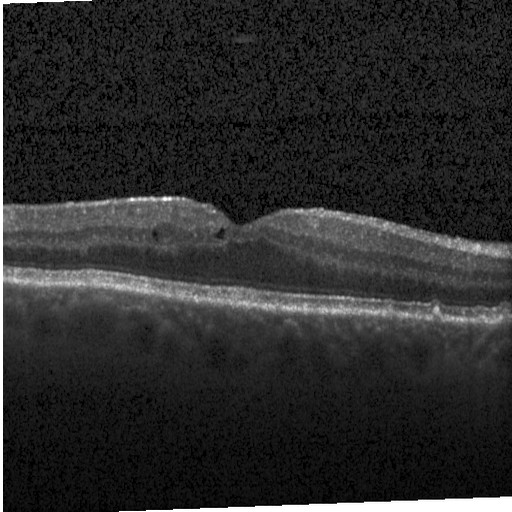 Diagnosis: DME.